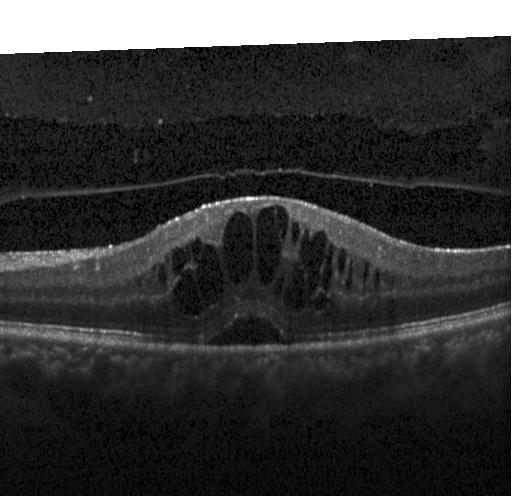
Retinal OCT B-scan — This B-scan demonstrates diabetic macular edema.